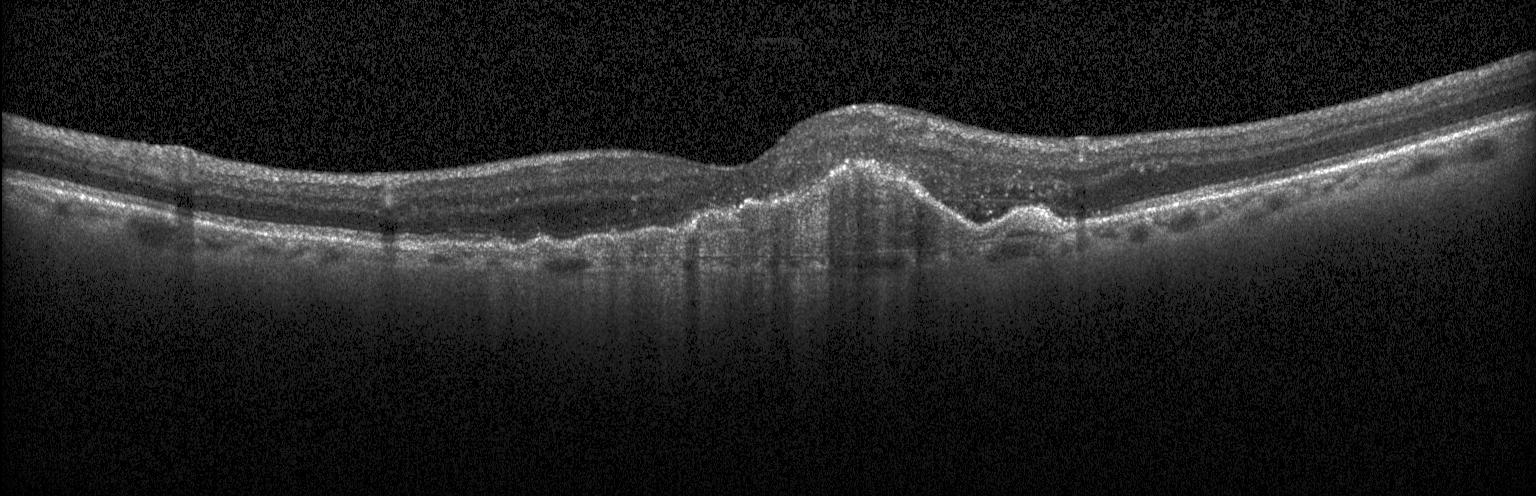 Fovea-centered · instrument: Heidelberg Spectralis · optical coherence tomography scan · spectral-domain OCT.
A choroidal neovascular membrane.